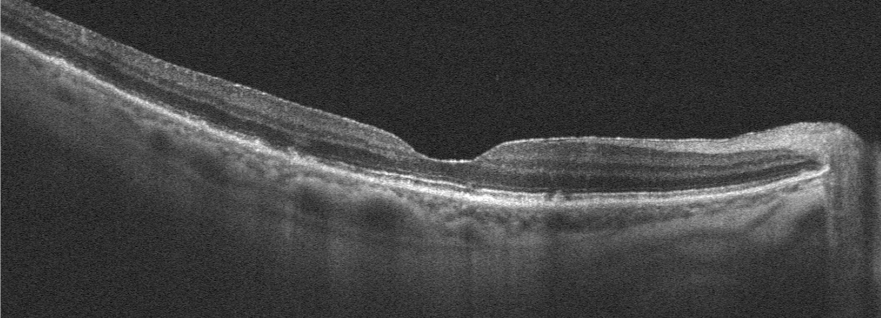
OCT scan showing AMD.